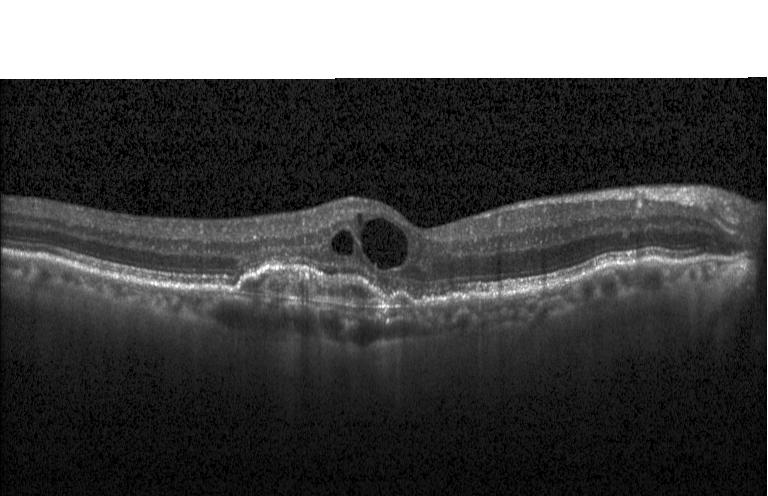
OCT B-scan. Assessment: a choroidal neovascular membrane.